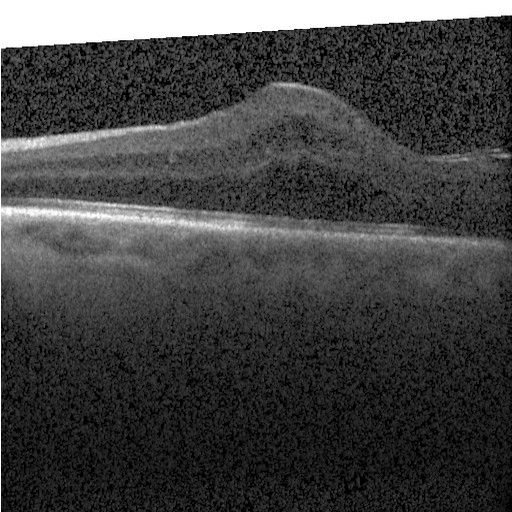
Diagnosis: diabetic macular edema (DME).